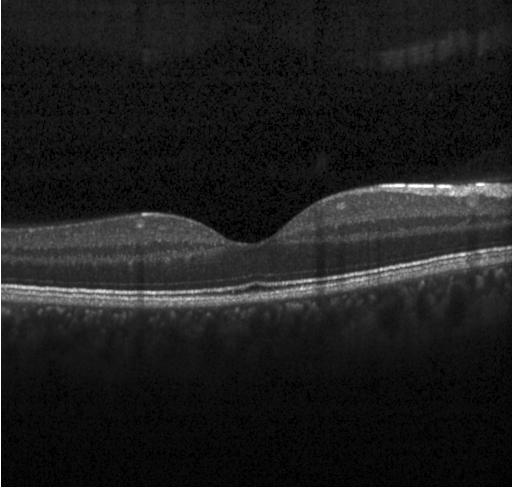
Retinal OCT cross-section.
Assessment: no CNV, DME, or drusen.